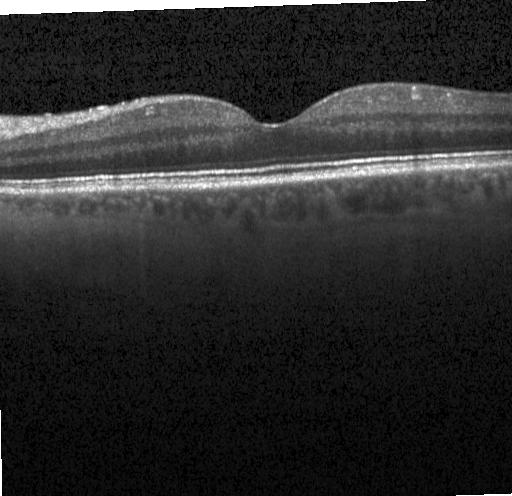
Horizontal scan through the fovea; OCT B-scan
Macular OCT: neither CNV, DME, nor drusen.